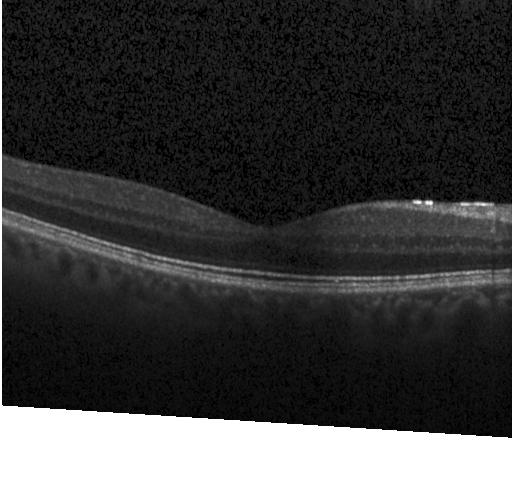
Optical coherence tomography scan.
Diagnosis: no choroidal neovascularization, no diabetic macular edema, and no drusen.